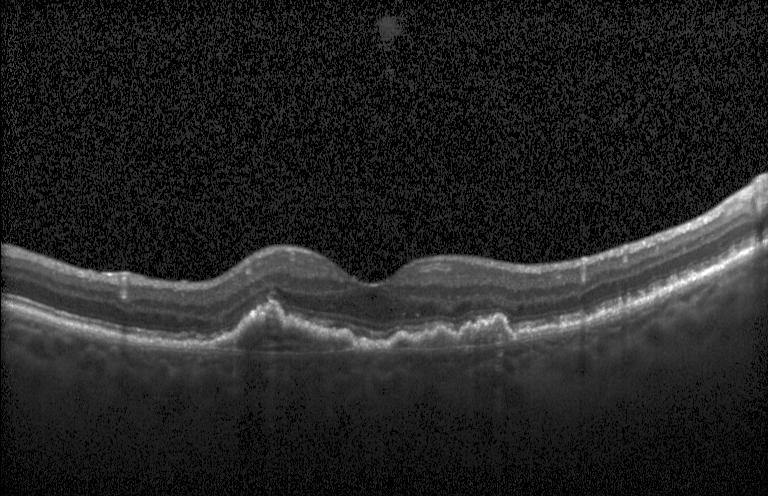

Optical coherence tomography B-scan. OCT finding: choroidal neovascularization (CNV).